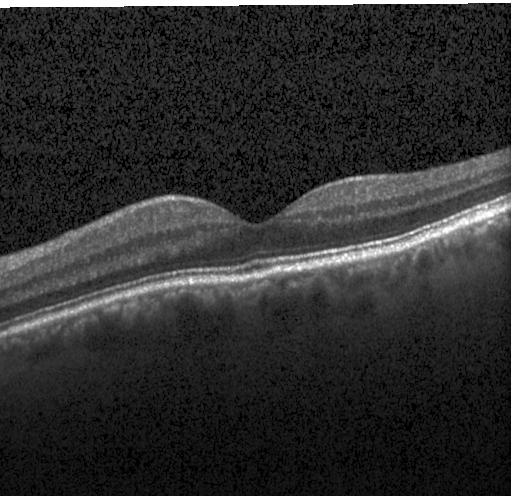

OCT scan showing no evidence of choroidal neovascularization, diabetic macular edema, or drusen.